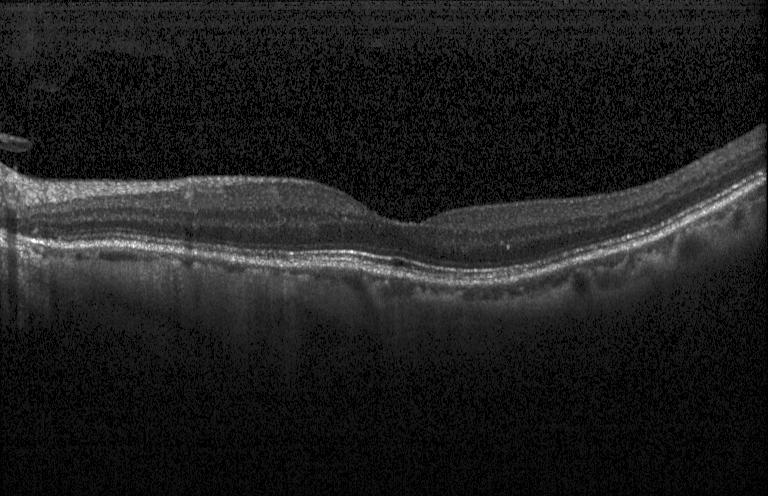
Optical coherence tomography B-scan; Heidelberg Spectralis.
Finding: no evidence of choroidal neovascularization, diabetic macular edema, or drusen.